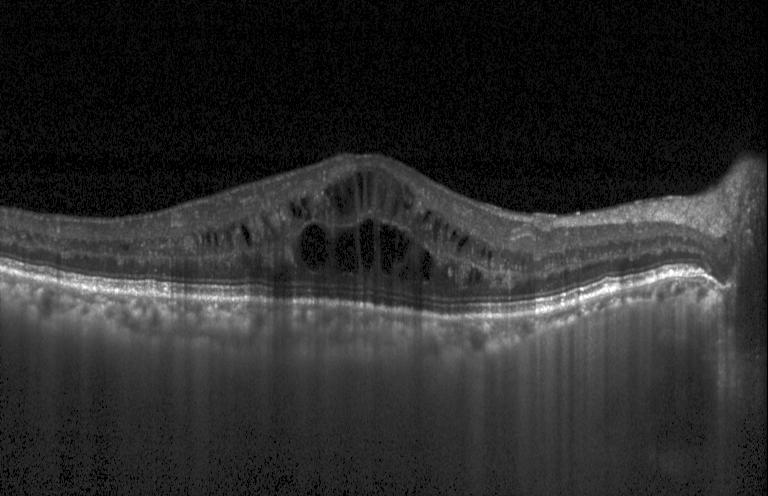
OCT B-scan showing diabetic macular edema (DME).